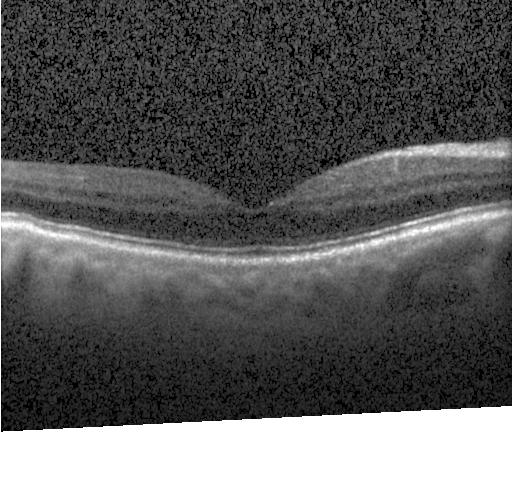
Macular OCT demonstrating no choroidal neovascularization, diabetic macular edema, or drusen.